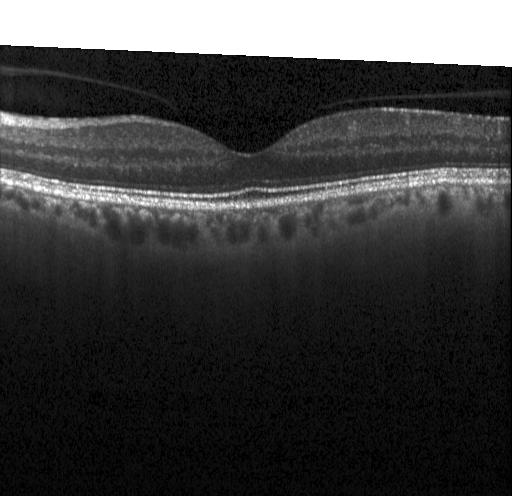

OCT finding: no evidence of choroidal neovascularization, diabetic macular edema, or drusen.